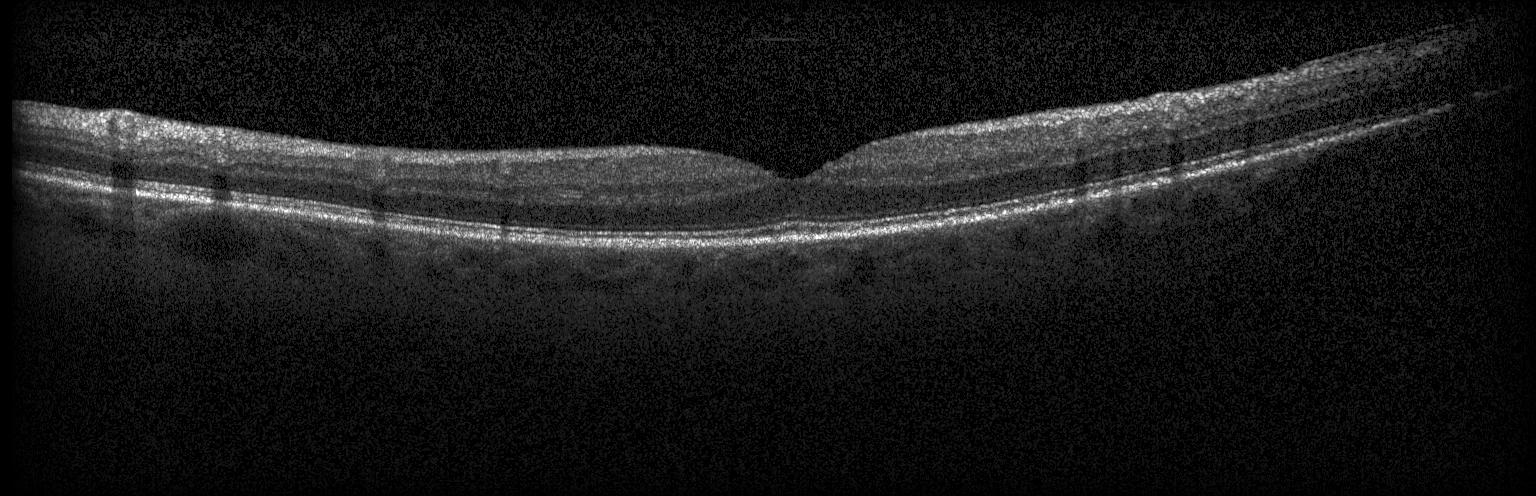
Diagnosis: no evidence of CNV, DME, or drusen.